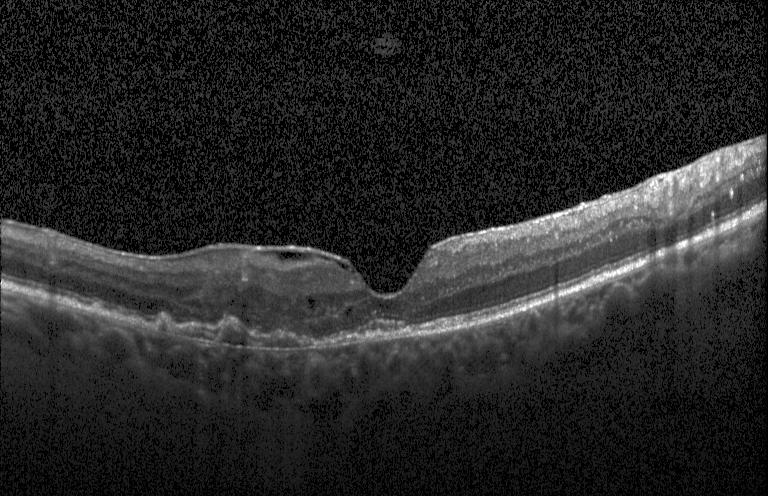 Optical coherence tomography scan — CNV.